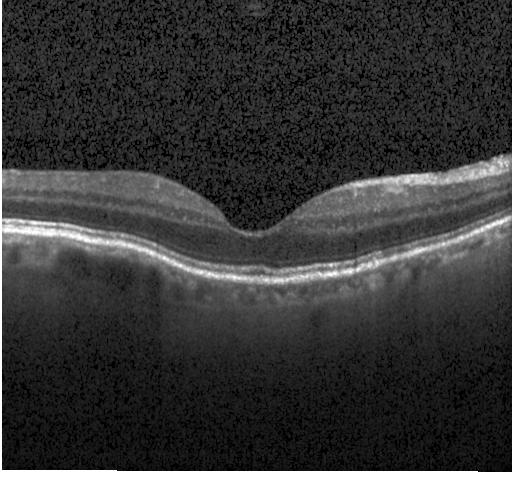

Through the macula; OCT line scan; acquired on a Heidelberg Spectralis.
Finding: no CNV, DME, or drusen.